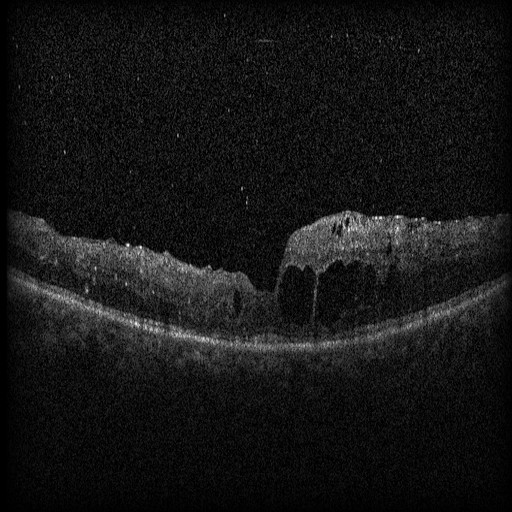

Heidelberg Spectralis. Macular scan. Spectral-domain OCT. Optical coherence tomography B-scan.
Impression: diabetic macular edema.